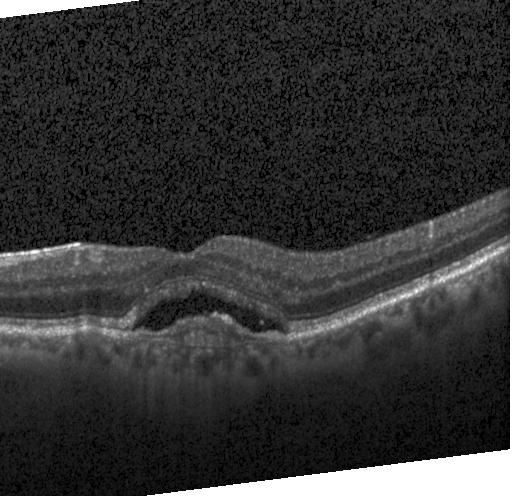 OCT line scan
The scan shows a choroidal neovascular membrane.